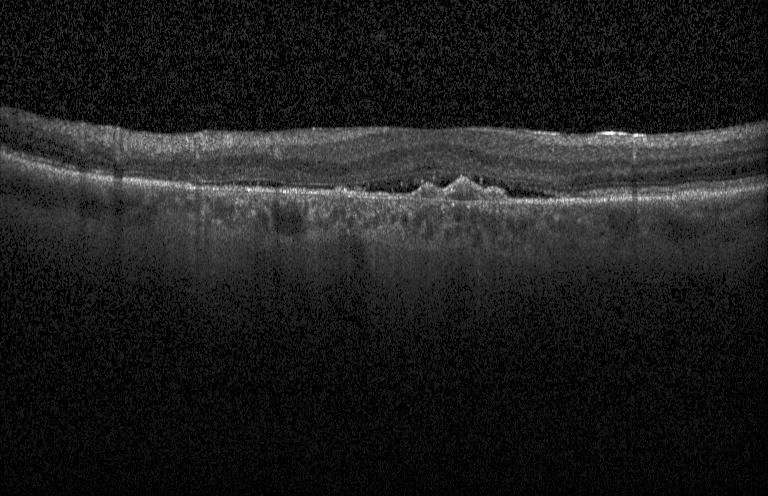
Impression: choroidal neovascularization (CNV).